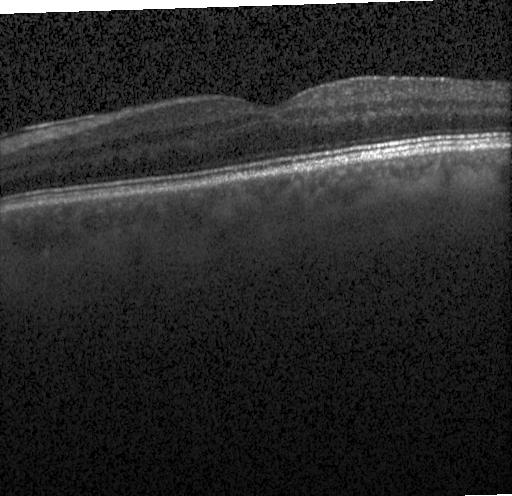
Spectral-domain optical coherence tomography · Heidelberg Spectralis OCT system · optical coherence tomography B-scan.
Macular OCT: no choroidal neovascularization, diabetic macular edema, or drusen.